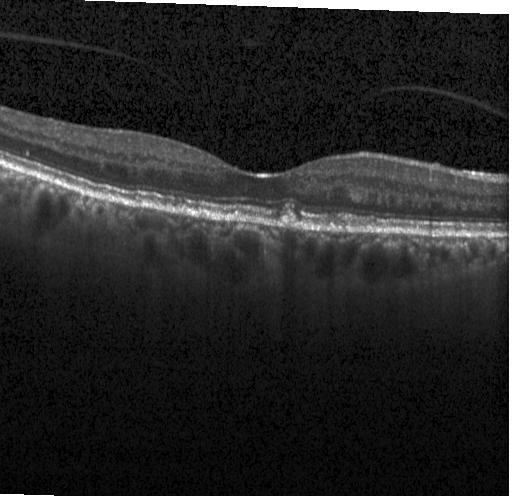
Diagnosis: drusen.